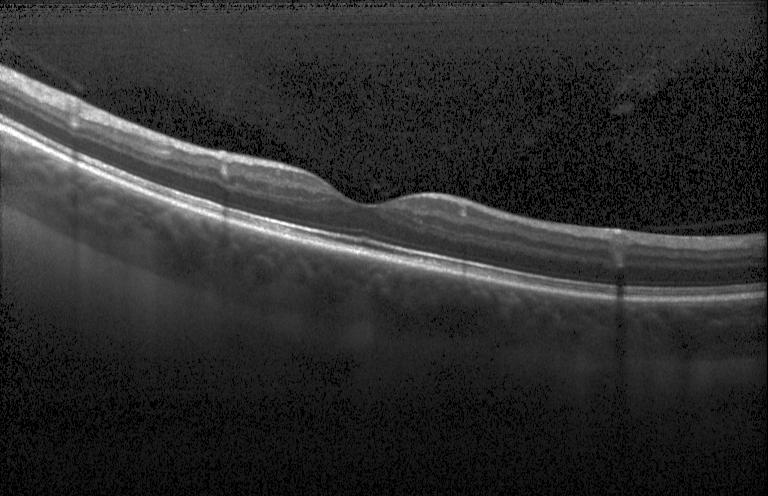 Optical coherence tomography scan; through the macula. OCT finding: no evidence of choroidal neovascularization, diabetic macular edema, or drusen.